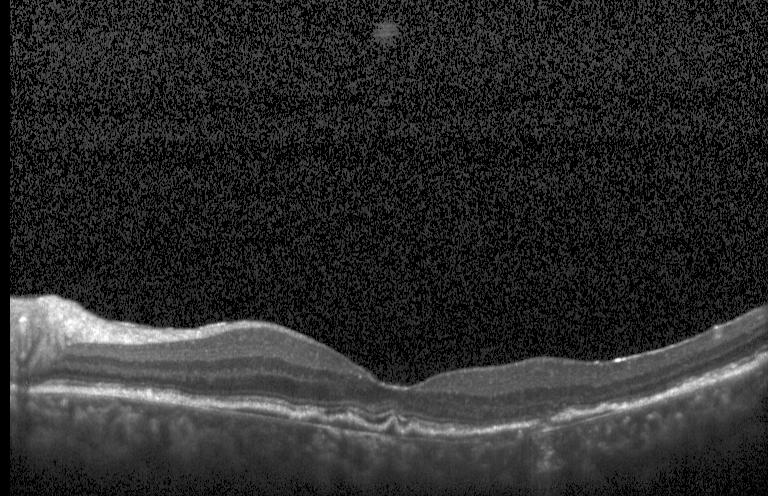

Impression: a choroidal neovascular membrane.